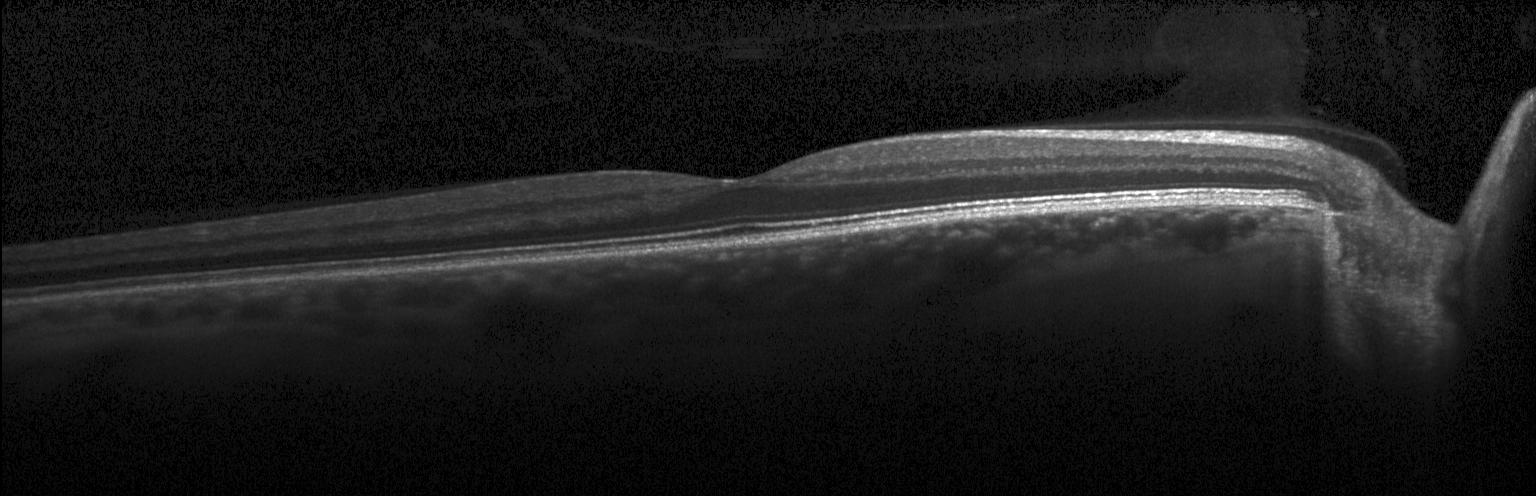

Optical coherence tomography B-scan
Diagnosis: neither CNV, DME, nor drusen.